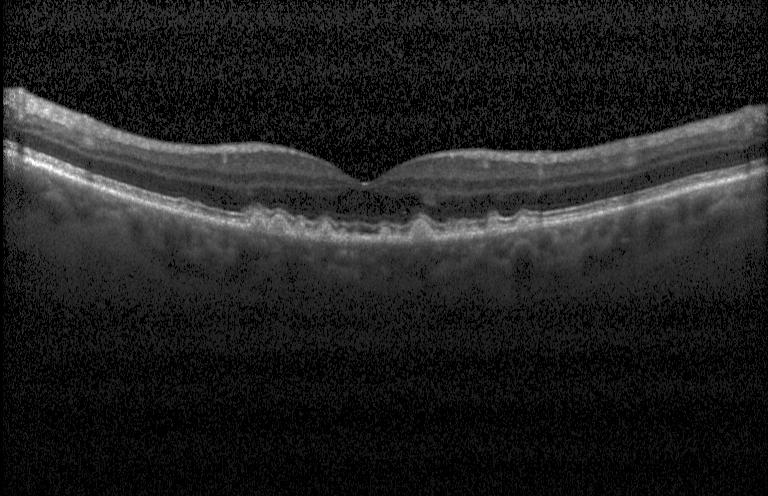

Retinal OCT cross-section showing multiple drusen.